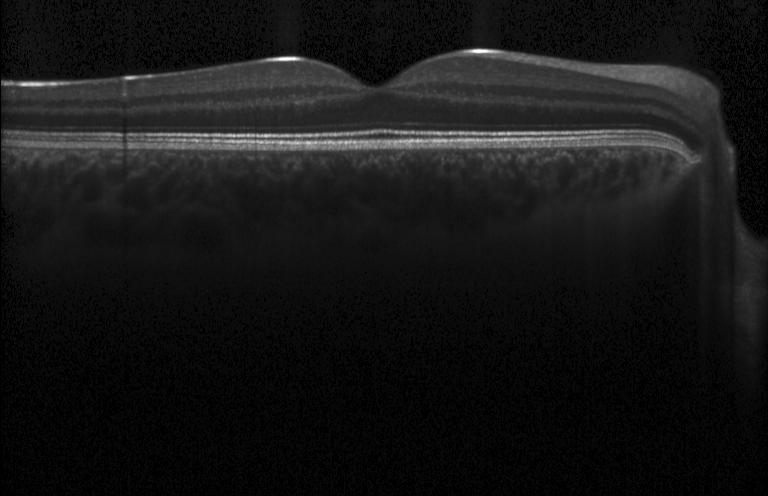

Fovea-centered, retinal OCT B-scan, spectral-domain optical coherence tomography
Impression: no choroidal neovascularization, diabetic macular edema, or drusen.